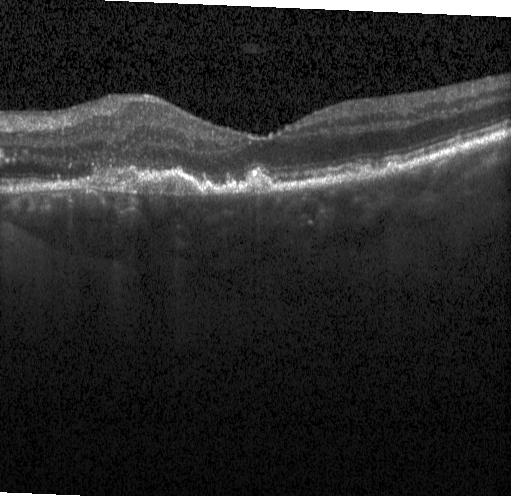

OCT B-scan · horizontal scan through the fovea.
Diagnosis: choroidal neovascularization (CNV).